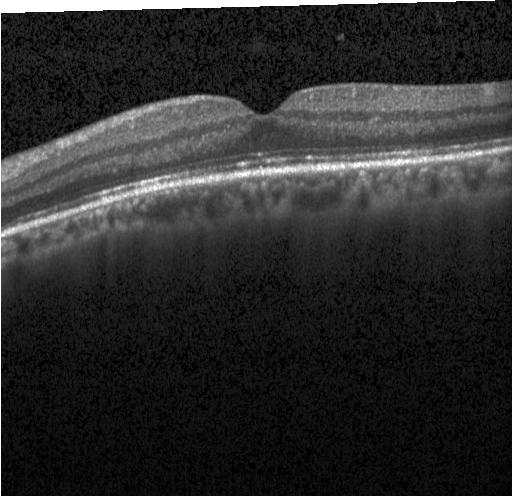

Diagnosis: no CNV, no DME, and no drusen.